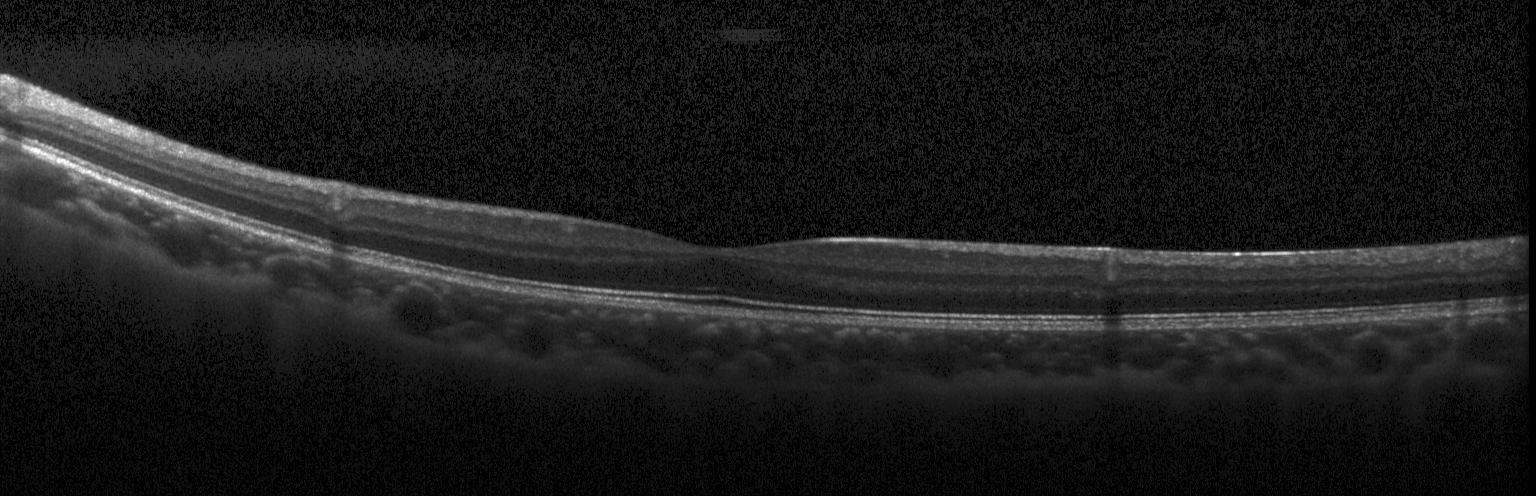
Optical coherence tomography B-scan — OCT finding: no choroidal neovascularization, diabetic macular edema, or drusen.